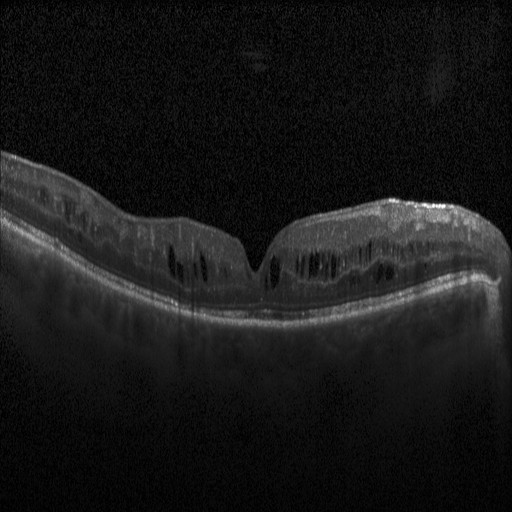

Spectral-domain OCT. Heidelberg Spectralis OCT system. OCT line scan. Centered on the fovea — Diabetic macular edema.